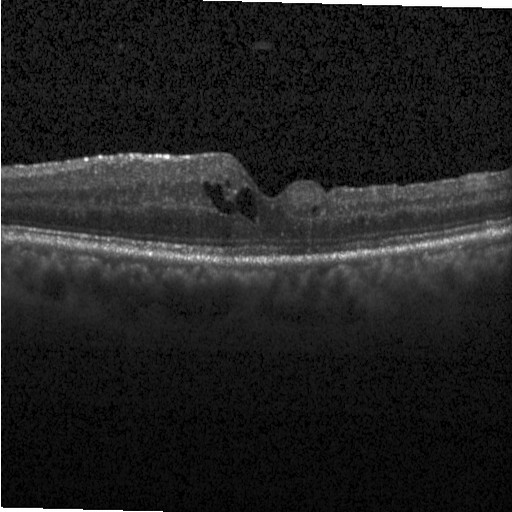
This B-scan demonstrates diabetic macular edema.